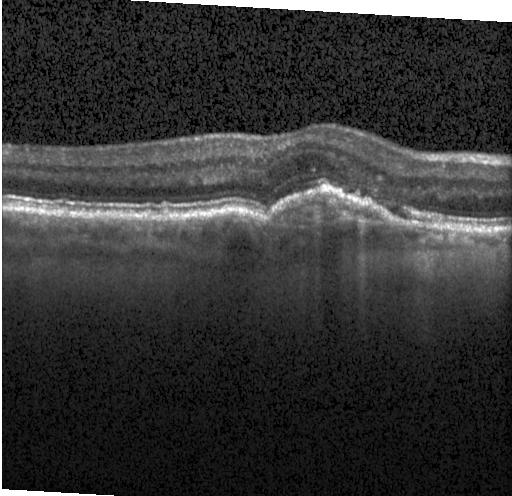

Acquired on a Heidelberg Spectralis, fovea-centered, spectral-domain OCT, OCT B-scan.
The scan shows CNV.